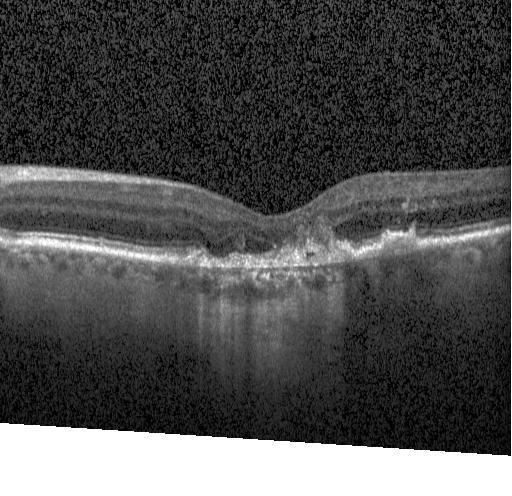
Impression: a choroidal neovascular membrane.